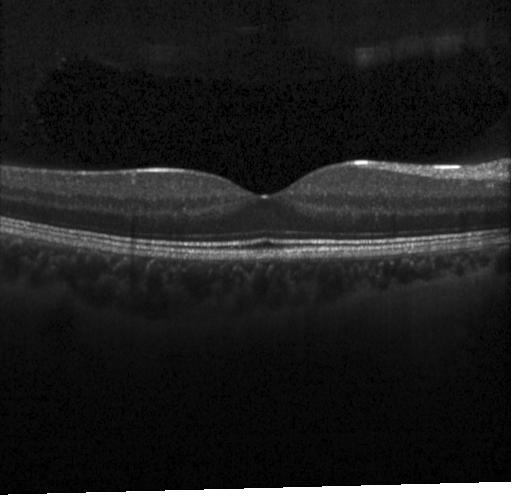

Diagnosis: neither choroidal neovascularization, diabetic macular edema, nor drusen.